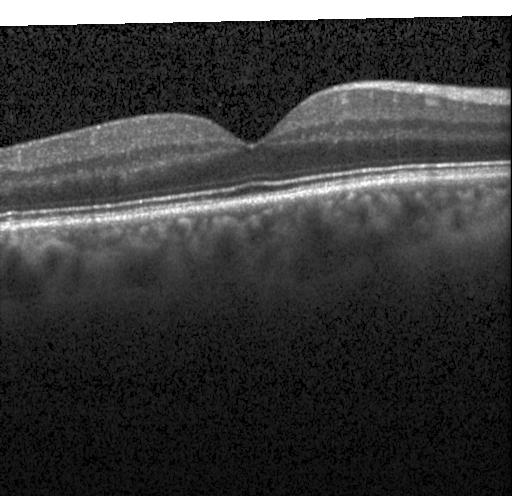
Retinal OCT B-scan
The scan shows no choroidal neovascularization, diabetic macular edema, or drusen.